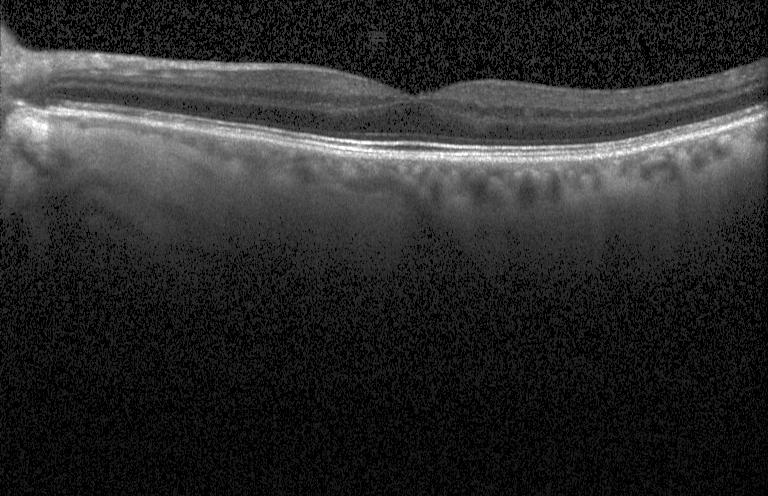
Horizontal scan through the fovea. OCT line scan. Heidelberg Spectralis. Spectral-domain optical coherence tomography. This B-scan demonstrates neither choroidal neovascularization, diabetic macular edema, nor drusen.